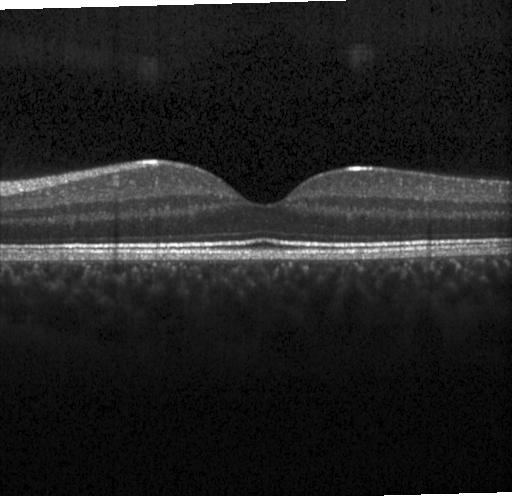 Finding: no choroidal neovascularization, no diabetic macular edema, and no drusen.